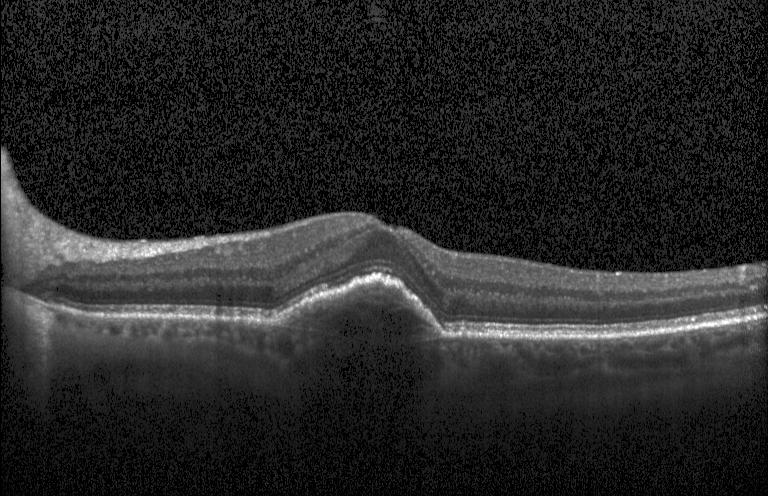

Spectral-domain OCT; Heidelberg Spectralis OCT system; retinal OCT B-scan; macular scan.
Diagnosis: choroidal neovascularization (CNV).